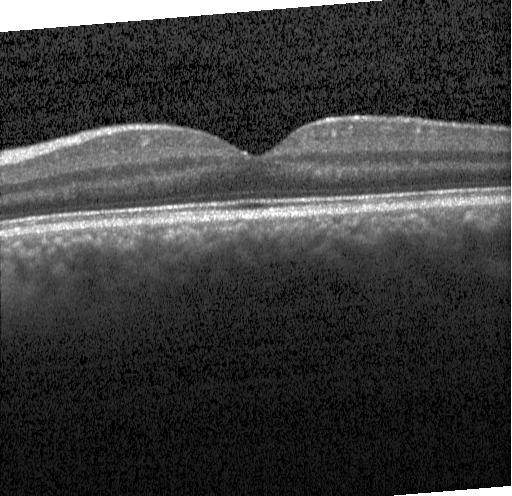

Diagnosis: neither choroidal neovascularization, diabetic macular edema, nor drusen.